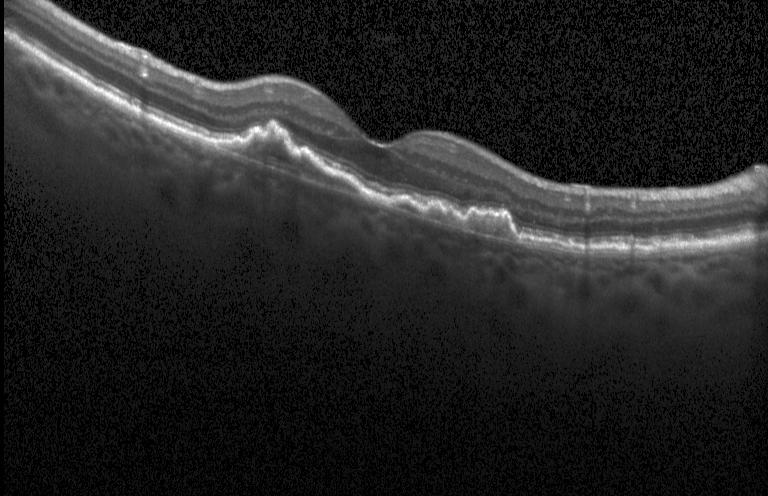

Fovea-centered; optical coherence tomography B-scan; spectral-domain OCT.
A choroidal neovascular membrane.